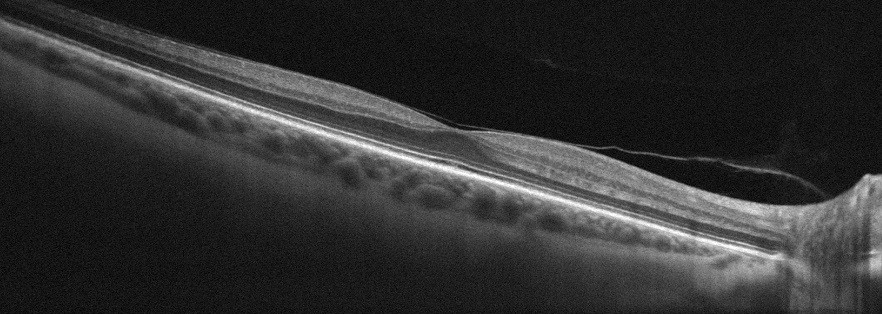

Through the macula. OCT B-scan. Acquired on an Optovue Avanti RTVue XR
Macular OCT: no evidence of AMD, DME, ERM, RAO, RVO, or VID.